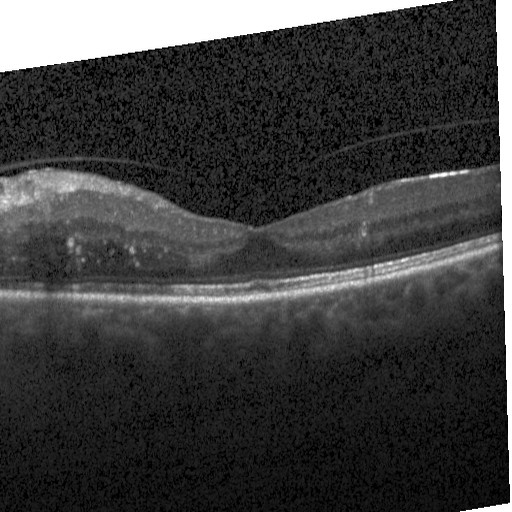
Through the macula · spectral-domain OCT · Heidelberg Spectralis · optical coherence tomography scan
Finding: diabetic macular edema.